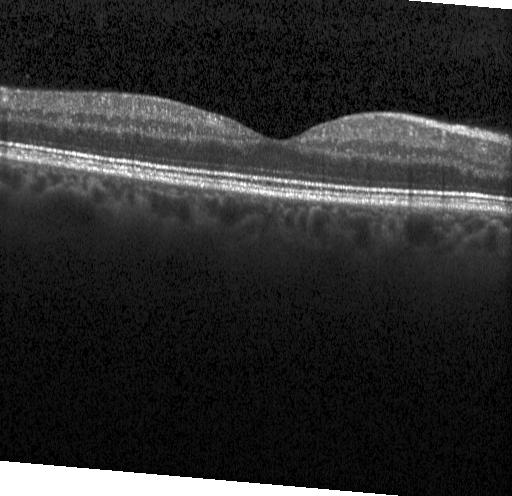
Optical coherence tomography scan. This B-scan demonstrates neither choroidal neovascularization, diabetic macular edema, nor drusen.